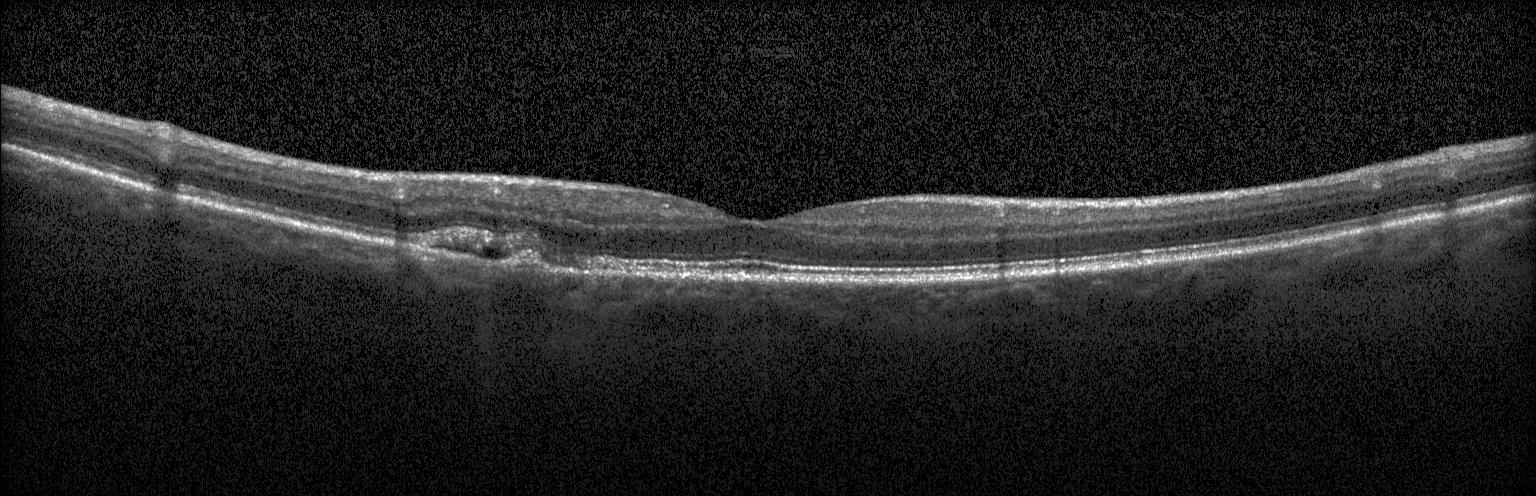 OCT line scan, SD-OCT. Finding: CNV.